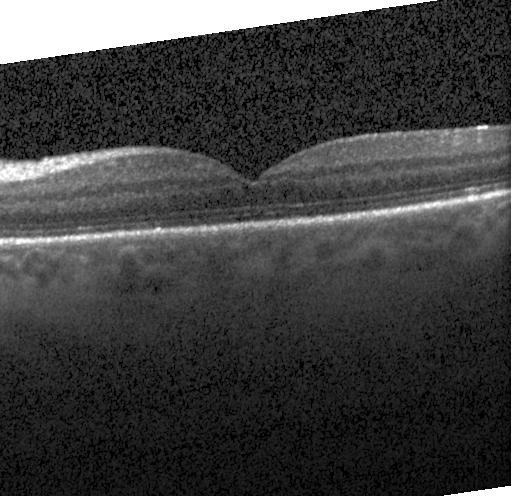

SD-OCT; fovea-centered; OCT B-scan; instrument: Heidelberg Spectralis. The scan shows no choroidal neovascularization, no diabetic macular edema, and no drusen.